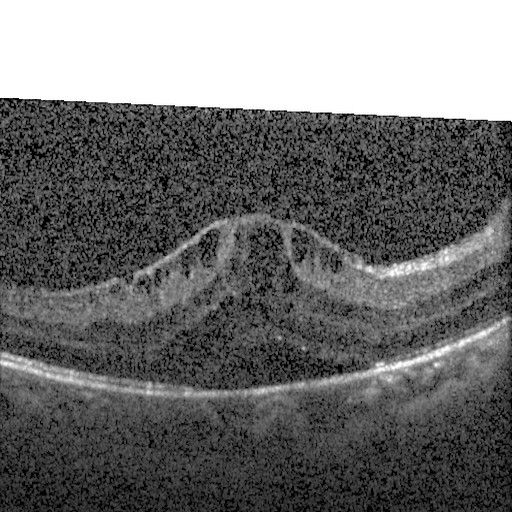

Macular OCT: DME.